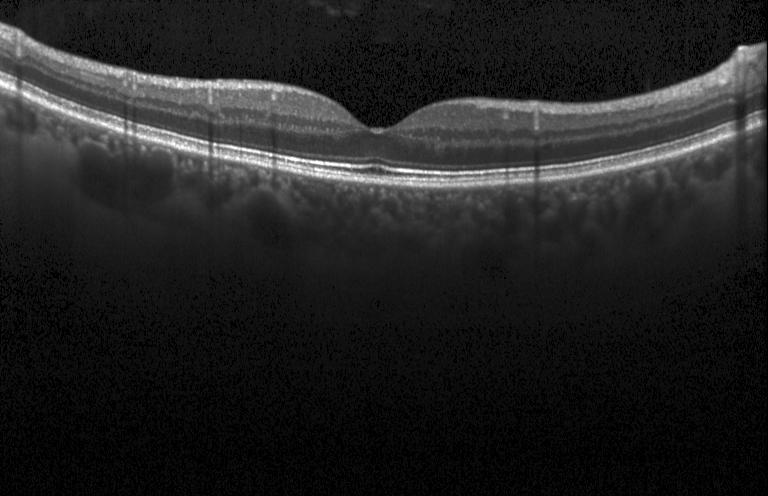
Heidelberg Spectralis OCT system · optical coherence tomography scan. Impression: no CNV, DME, or drusen.